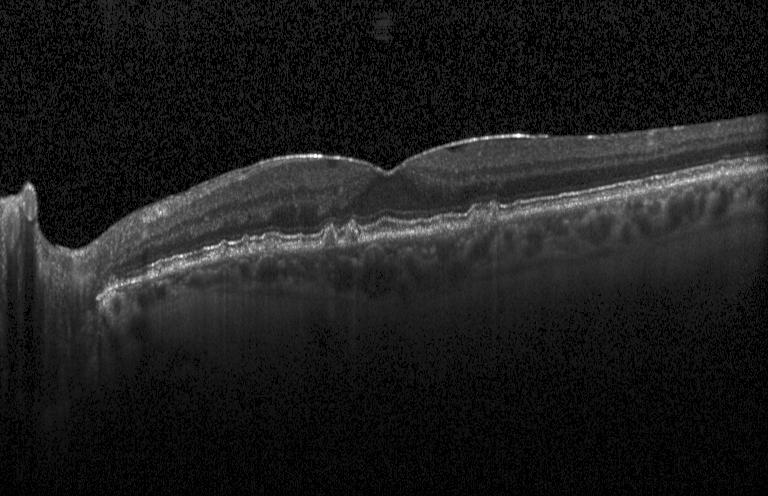

Through the macula, retinal OCT B-scan, SD-OCT.
Finding: sub-RPE drusenoid deposits.